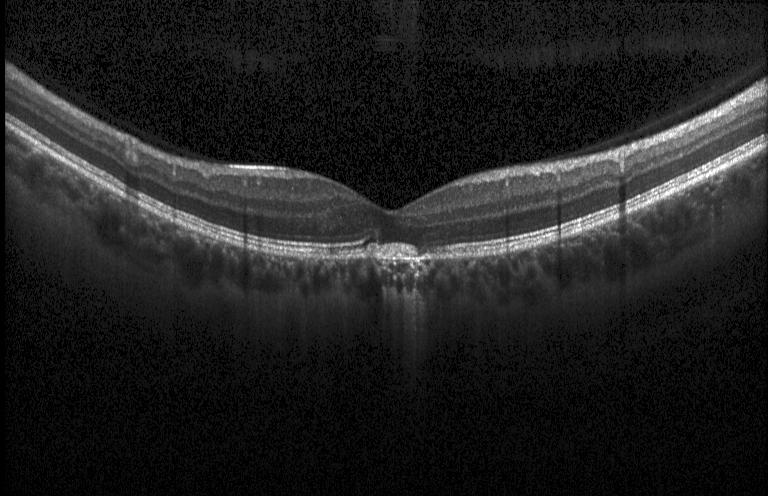

Heidelberg Spectralis; horizontal scan through the fovea; OCT B-scan.
Impression: choroidal neovascularization.